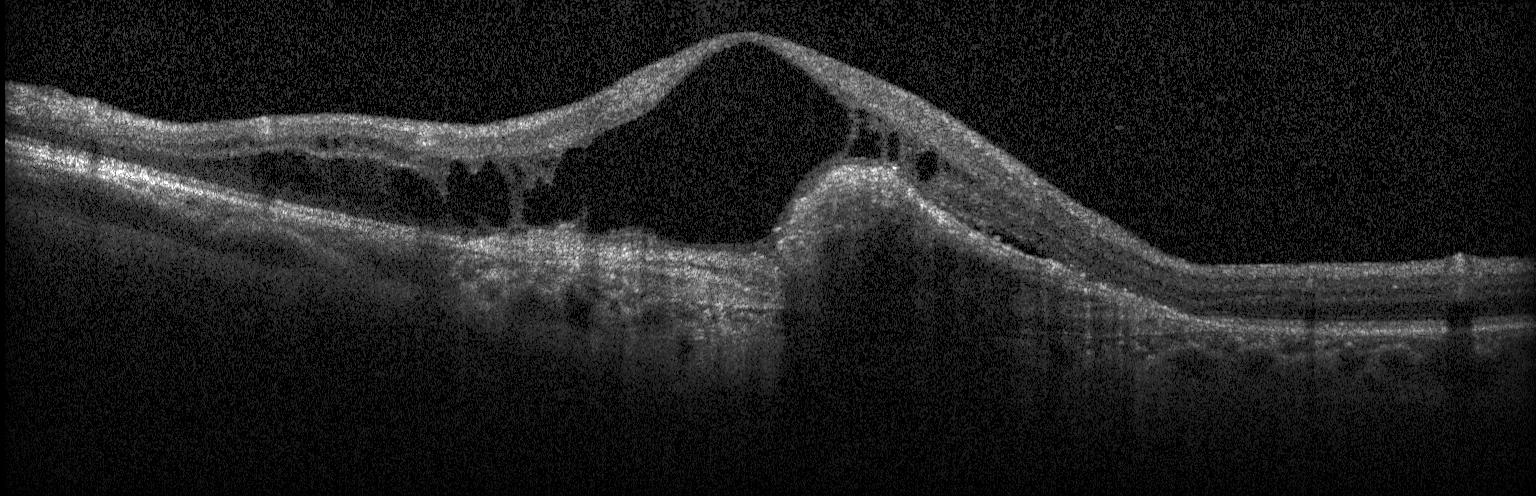
Spectral-domain OCT B-scan: choroidal neovascularization (CNV).